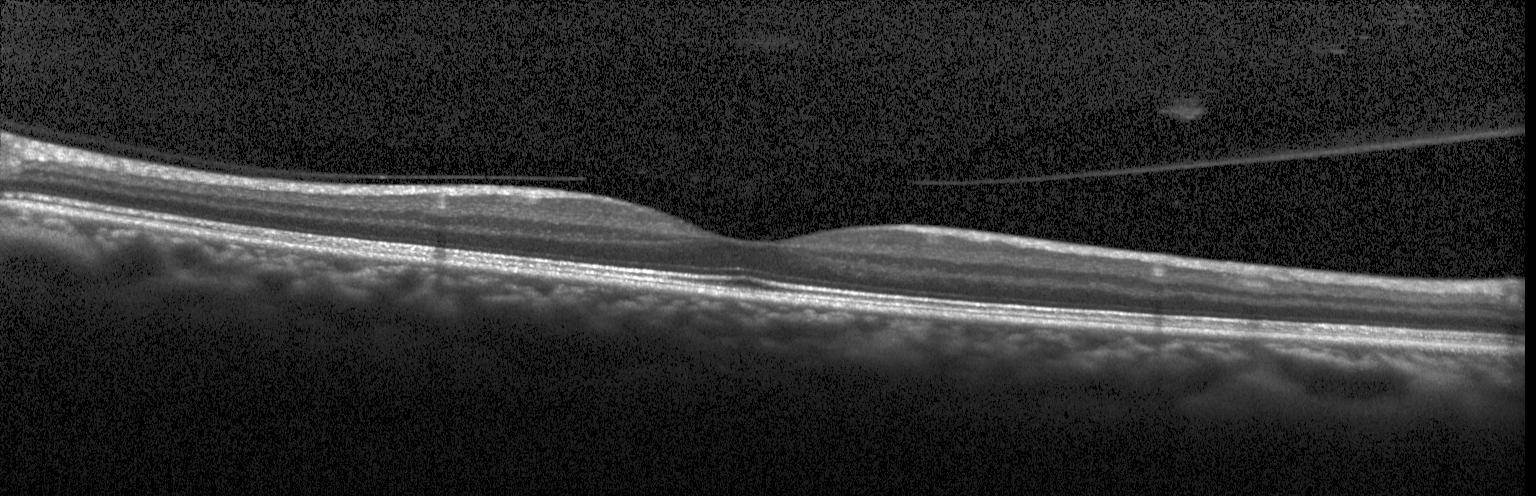
Optical coherence tomography B-scan. Impression: neither choroidal neovascularization, diabetic macular edema, nor drusen.